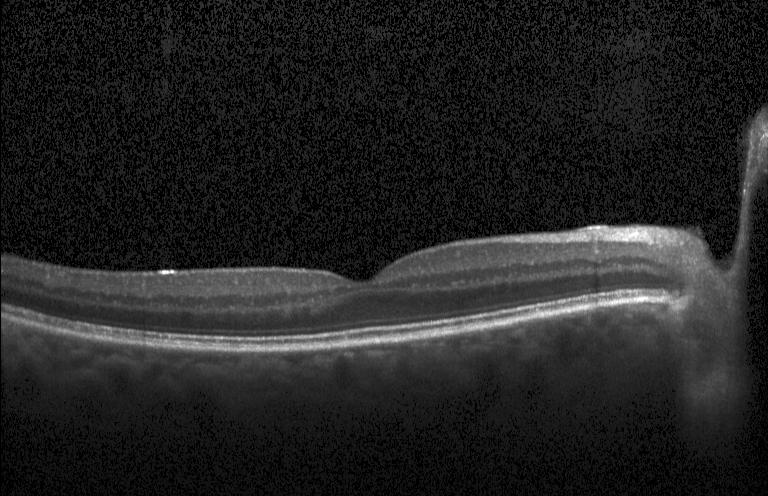 Impression: no evidence of choroidal neovascularization, diabetic macular edema, or drusen.